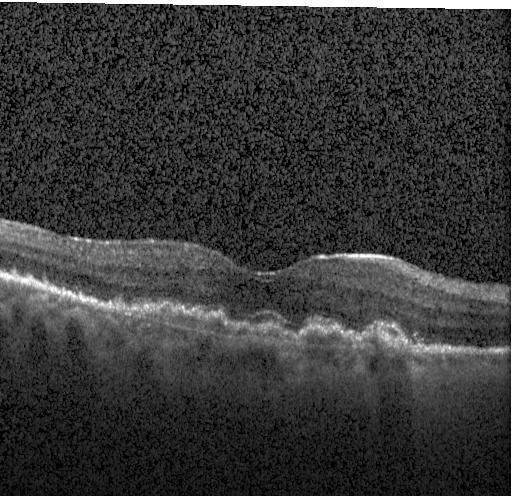

Impression: a choroidal neovascular membrane.